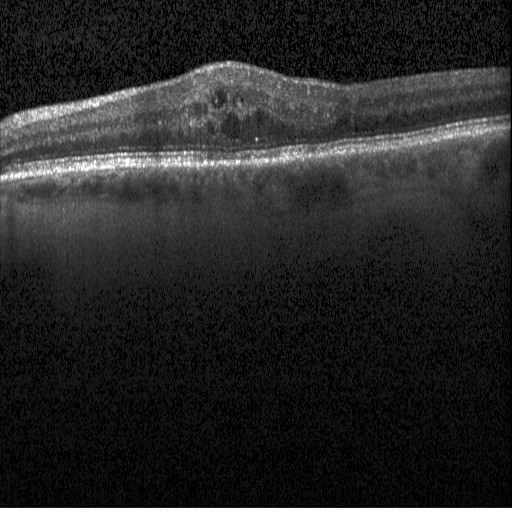

Dx: DME.